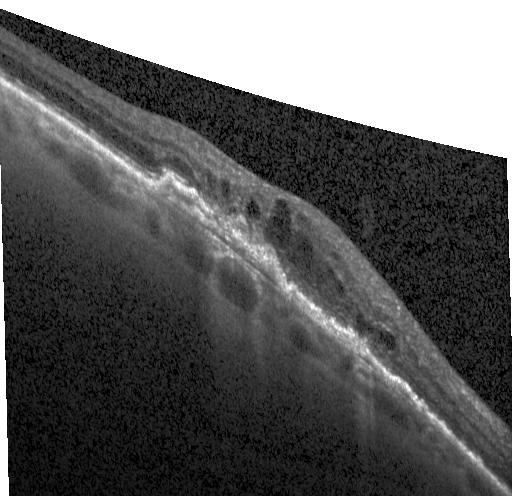
Impression: choroidal neovascularization.